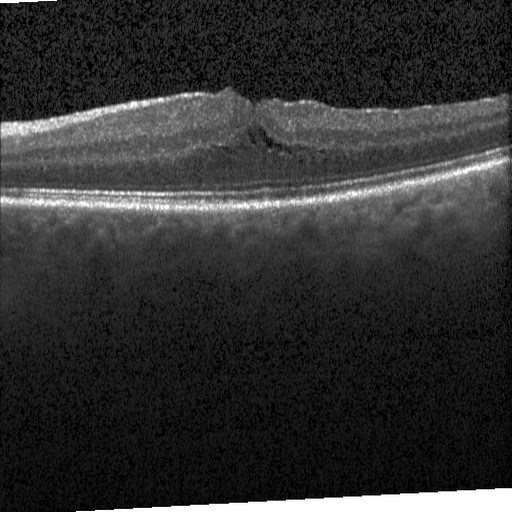
Retinal OCT B-scan. Impression: DME.